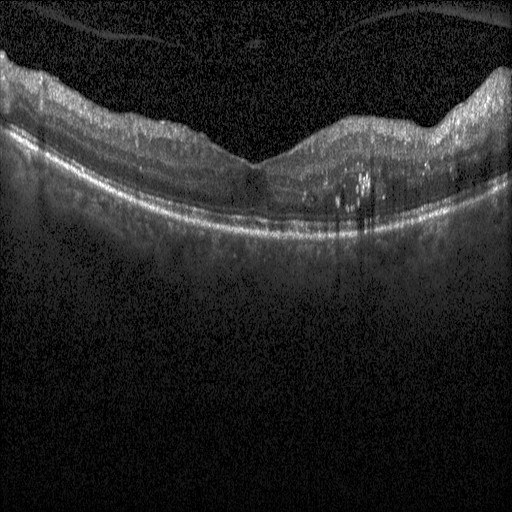 Retinal OCT B-scan · SD-OCT. Finding: diabetic macular edema (DME).